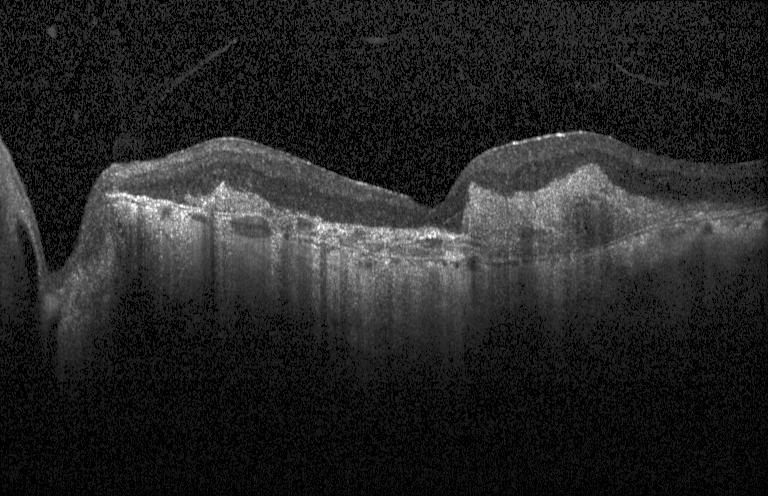
OCT B-scan. Spectral-domain optical coherence tomography. Acquired on a Heidelberg Spectralis — The scan shows choroidal neovascularization.